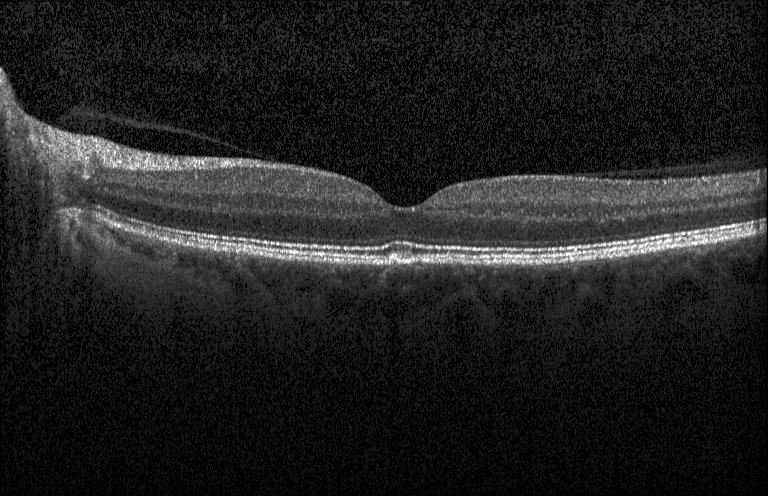 OCT finding: no choroidal neovascularization, no diabetic macular edema, and no drusen.